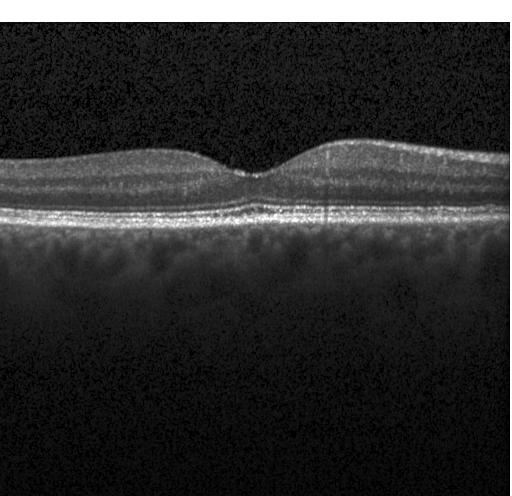 OCT line scan; centered on the fovea; instrument: Heidelberg Spectralis — Macular OCT: no evidence of choroidal neovascularization, diabetic macular edema, or drusen.